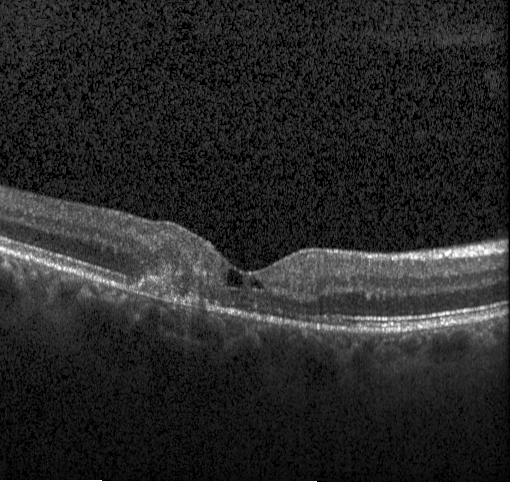 OCT B-scan; through the macula. Impression: a choroidal neovascular membrane.